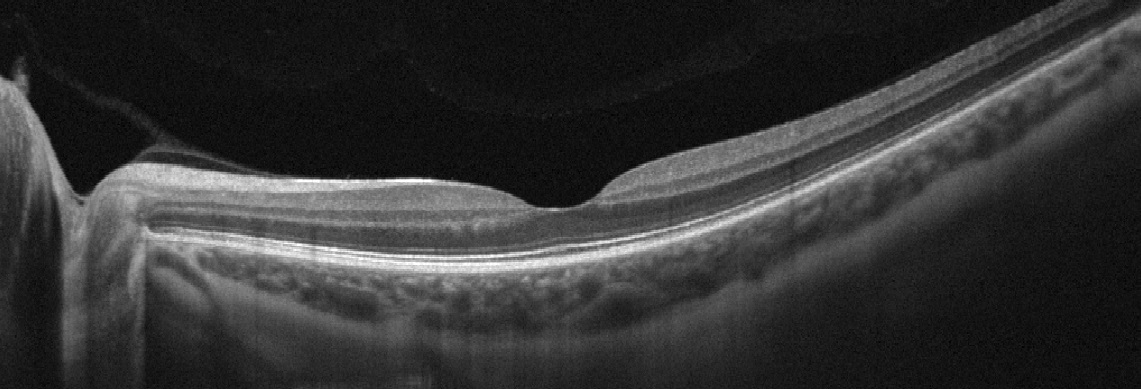

OCT line scan.
Impression: no evidence of AMD, DME, ERM, RAO, RVO, or VID.